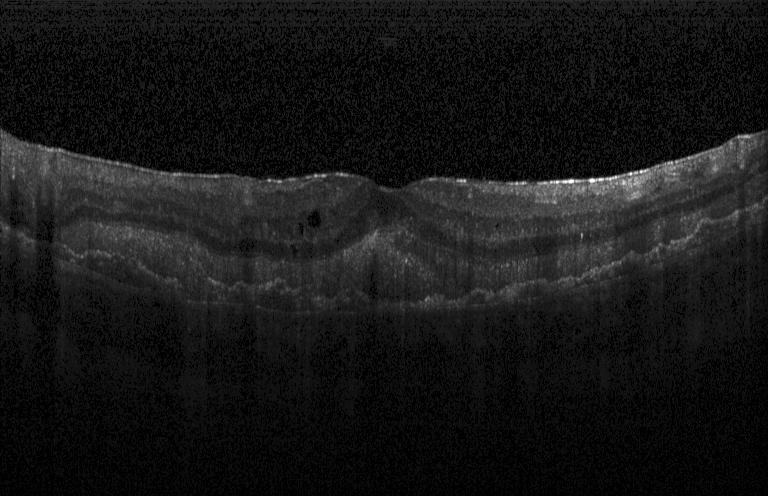 Impression: a choroidal neovascular membrane.